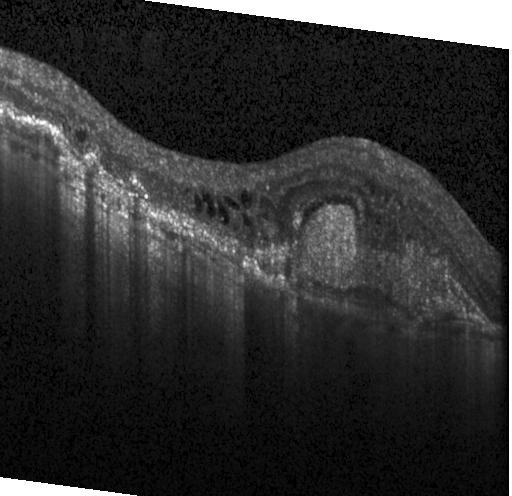 Diagnosis: a choroidal neovascular membrane.